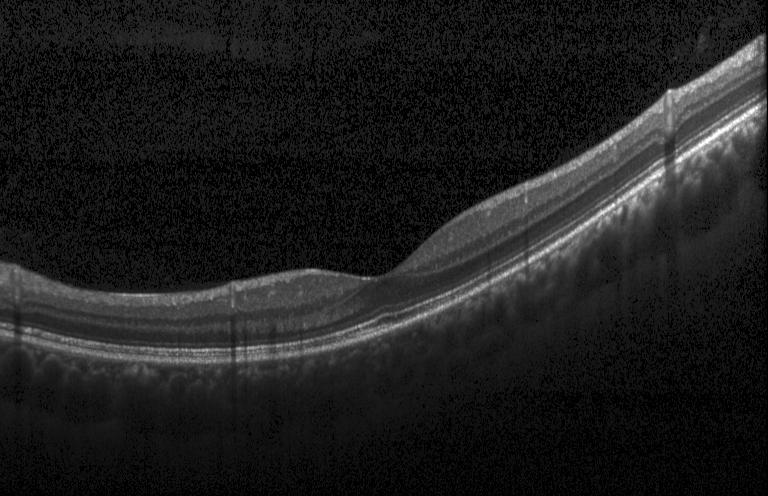

OCT line scan. Spectral-domain OCT.
Finding: no choroidal neovascularization, diabetic macular edema, or drusen.